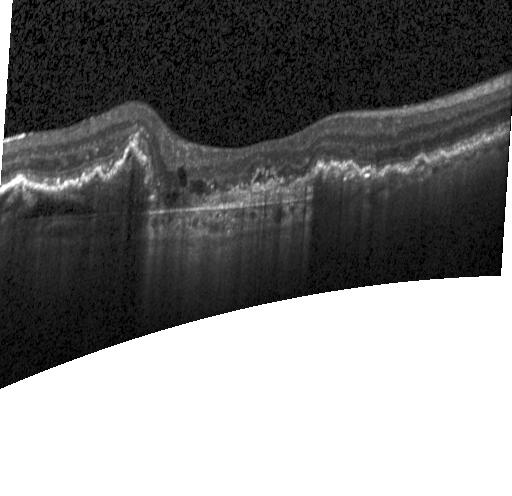
OCT B-scan; Heidelberg Spectralis.
Finding: a choroidal neovascular membrane.